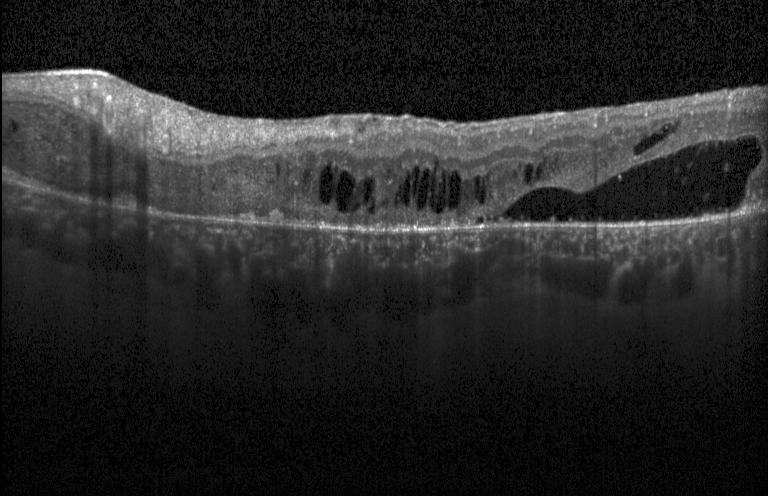
Optical coherence tomography B-scan — OCT finding: DME.